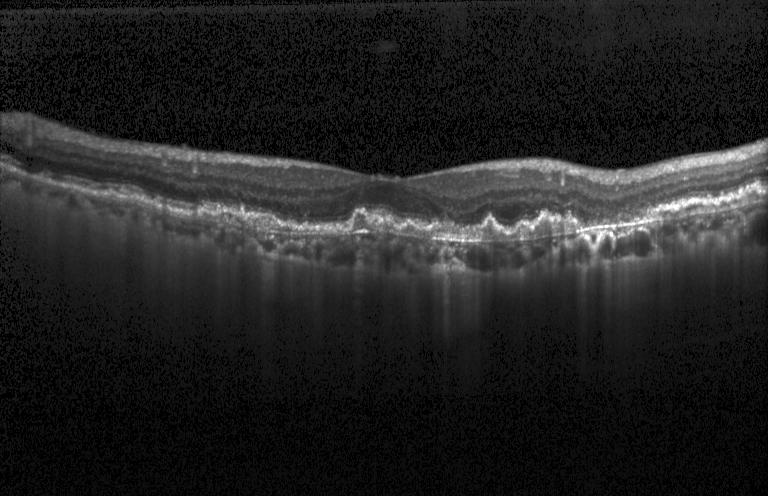 Instrument: Heidelberg Spectralis · retinal OCT B-scan · spectral-domain OCT.
Assessment: choroidal neovascularization (CNV).